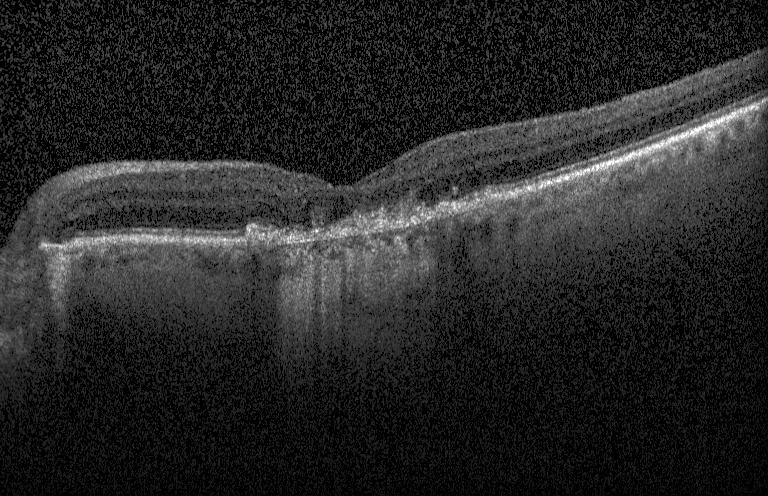 A choroidal neovascular membrane.